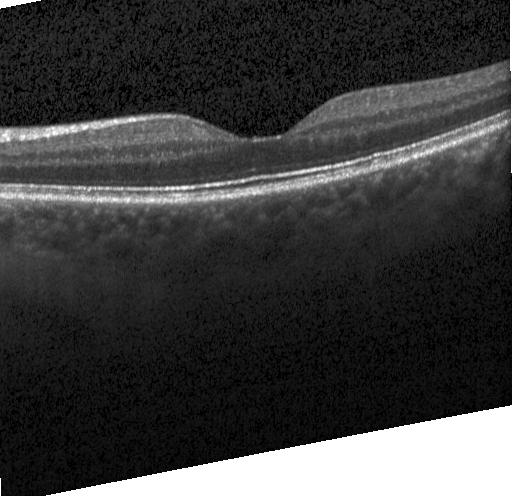 OCT line scan · fovea-centered · instrument: Heidelberg Spectralis.
OCT finding: no choroidal neovascularization, diabetic macular edema, or drusen.